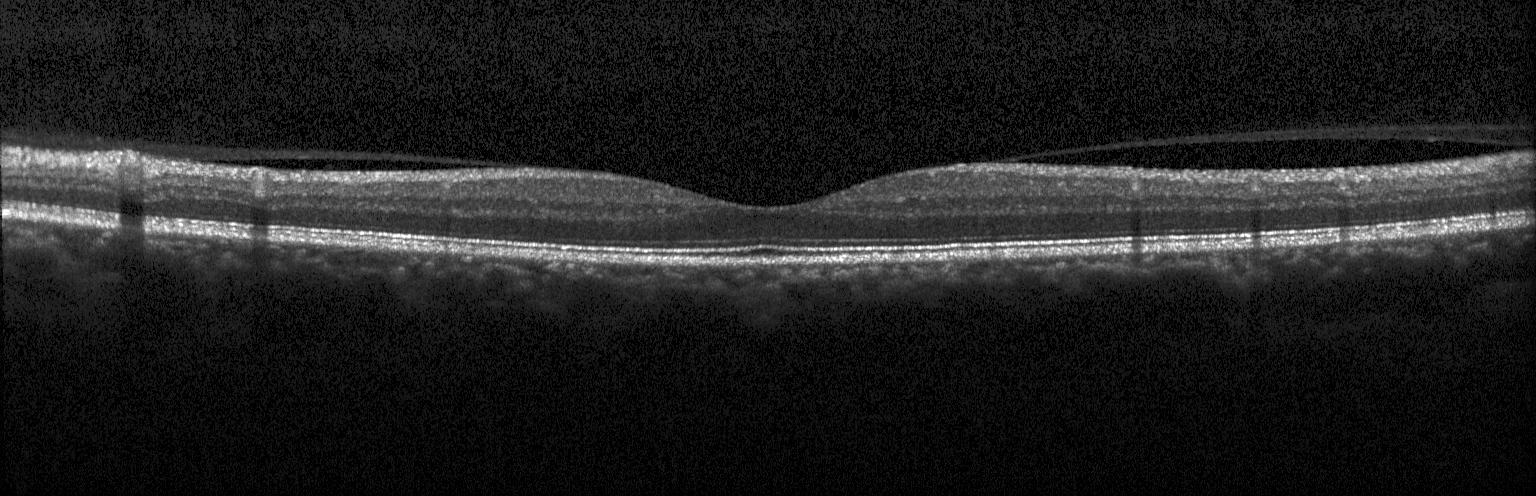

Acquired on a Heidelberg Spectralis · spectral-domain optical coherence tomography · OCT line scan. Impression: no choroidal neovascularization, no diabetic macular edema, and no drusen.